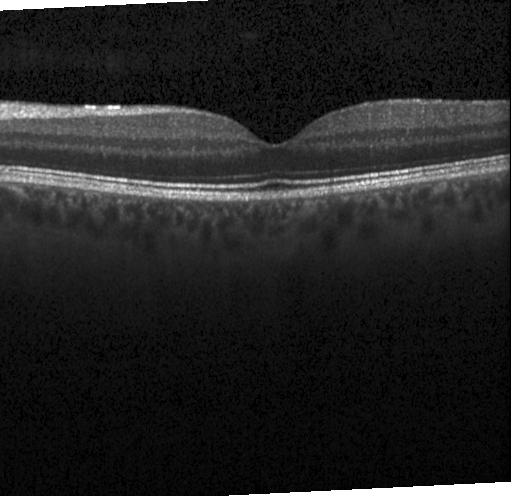

Optical coherence tomography B-scan · spectral-domain OCT · Heidelberg Spectralis · centered on the fovea — Finding: neither CNV, DME, nor drusen.